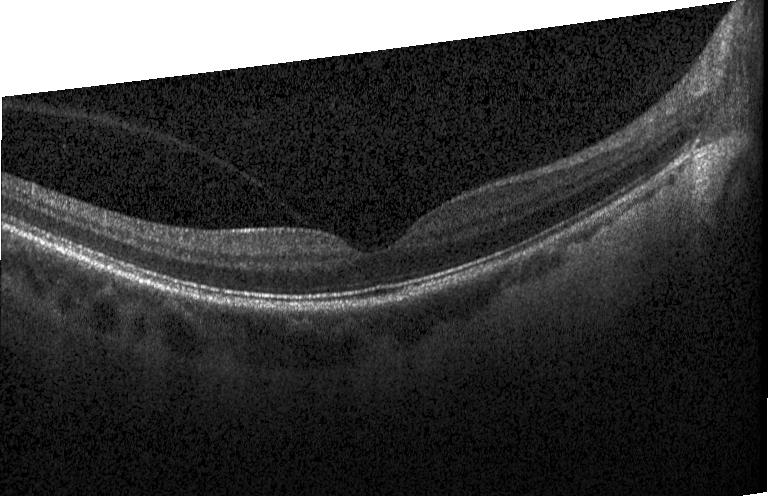

Retinal OCT B-scan · SD-OCT · centered on the fovea.
Impression: no choroidal neovascularization, no diabetic macular edema, and no drusen.